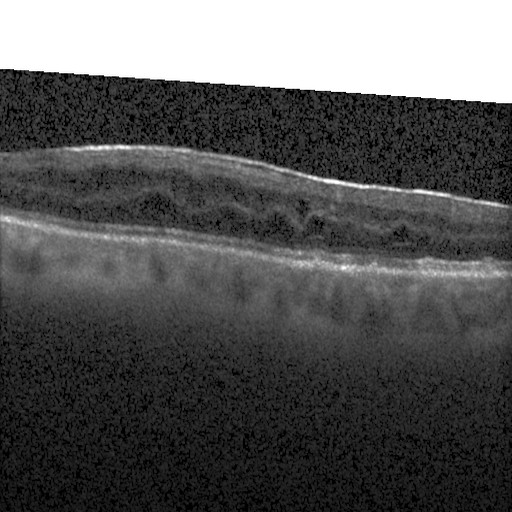
Diagnosis: diabetic macular edema (DME).